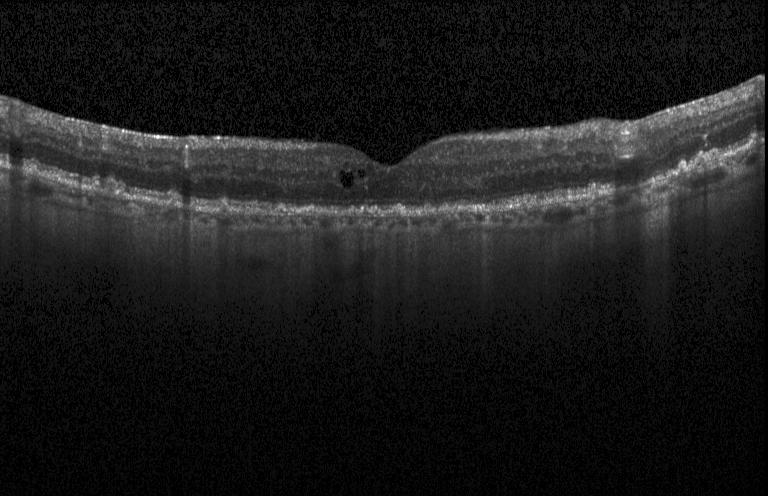

OCT line scan · Heidelberg Spectralis — OCT finding: choroidal neovascularization.